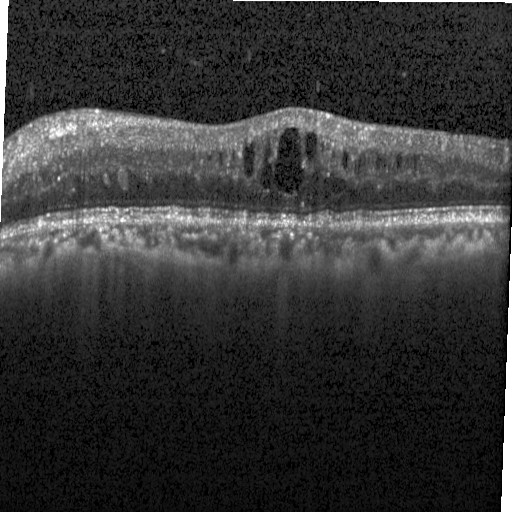 Fovea-centered · retinal OCT cross-section · Heidelberg Spectralis OCT system · spectral-domain OCT — Impression: diabetic macular edema (DME).